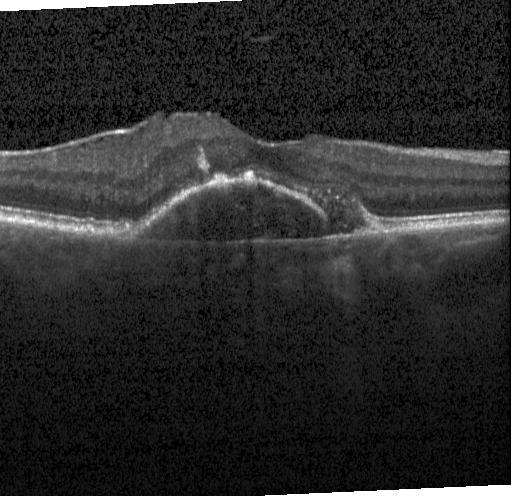
Optical coherence tomography scan · spectral-domain optical coherence tomography · instrument: Heidelberg Spectralis
OCT finding: a choroidal neovascular membrane.